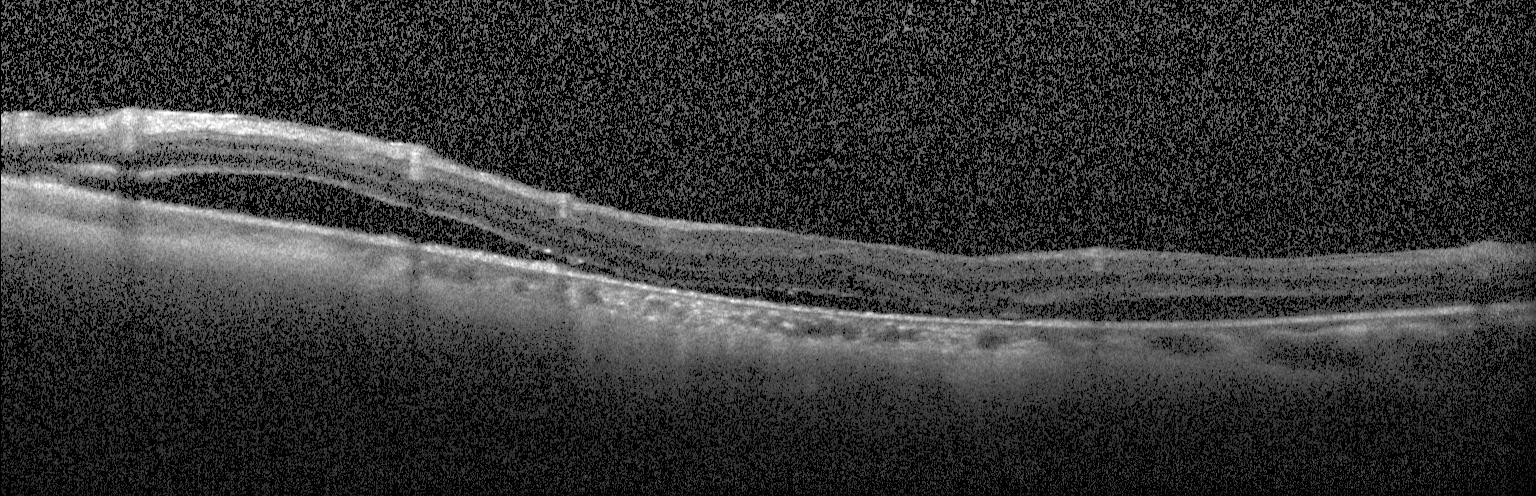
Through the macula · retinal OCT cross-section — OCT finding: CNV.